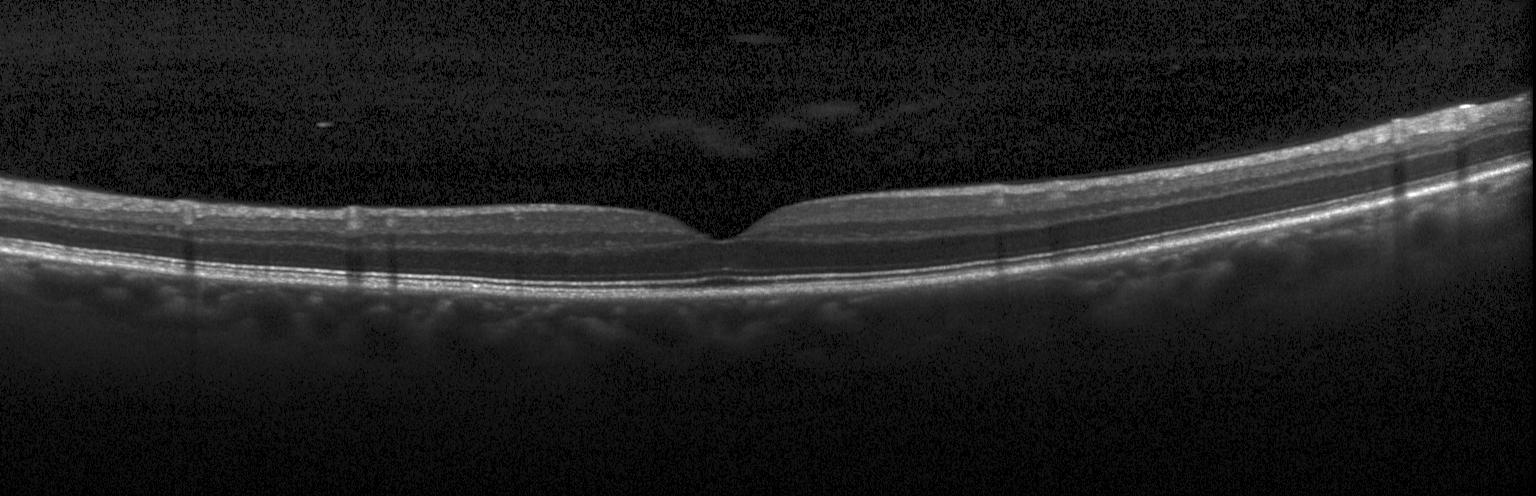

Fovea-centered; Heidelberg Spectralis; optical coherence tomography scan.
Impression: no evidence of choroidal neovascularization, diabetic macular edema, or drusen.